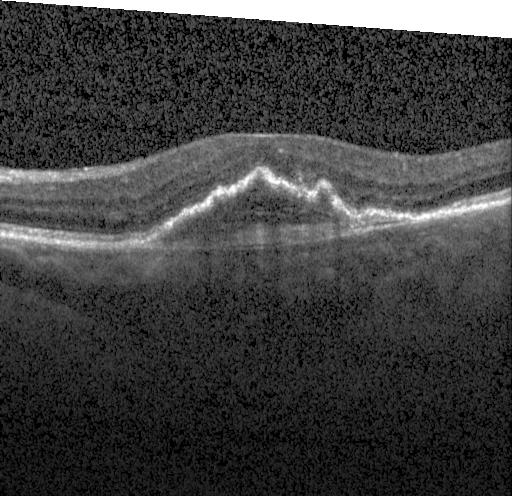

Horizontal scan through the fovea; SD-OCT; Heidelberg Spectralis; OCT line scan.
Finding: a choroidal neovascular membrane.